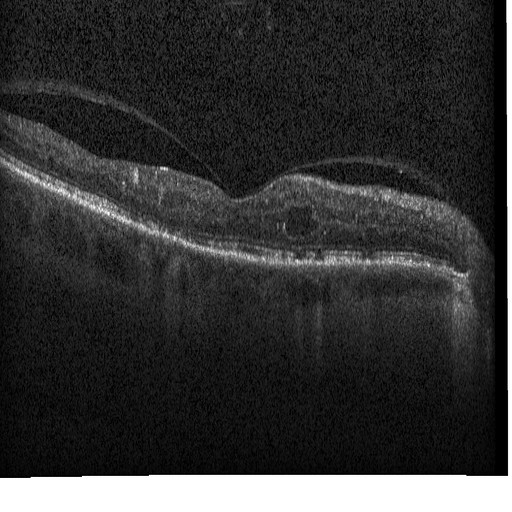 Spectral-domain OCT B-scan: DME.